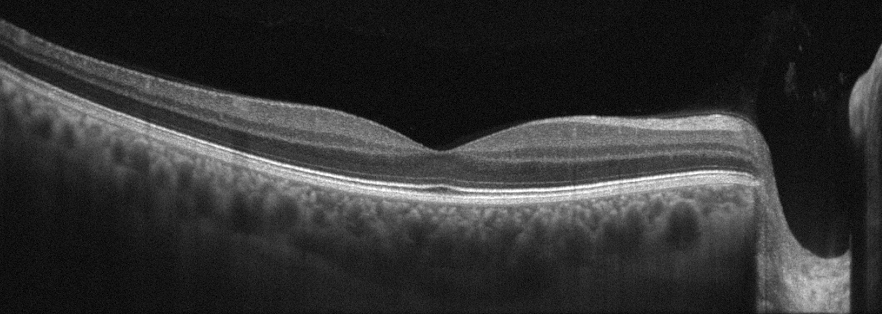 Right eye · optical coherence tomography scan.
OCT finding: no evidence of AMD, DME, ERM, RAO, RVO, or VID.